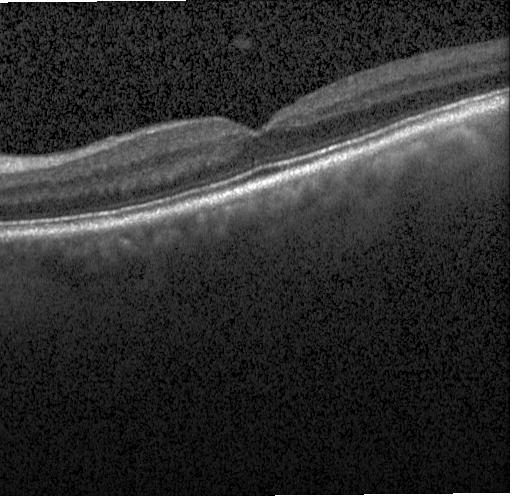 OCT line scan. Finding: neither choroidal neovascularization, diabetic macular edema, nor drusen.